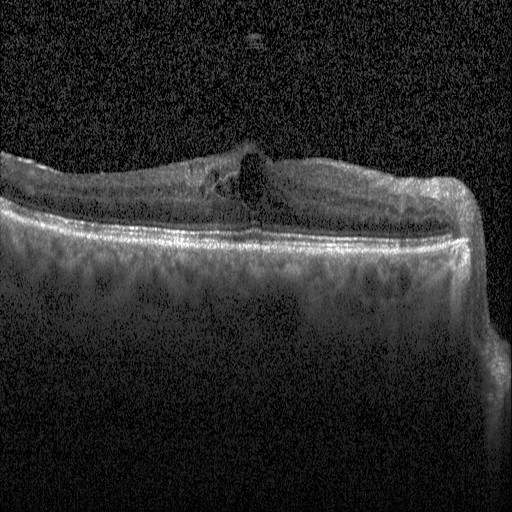

Finding: diabetic macular edema.